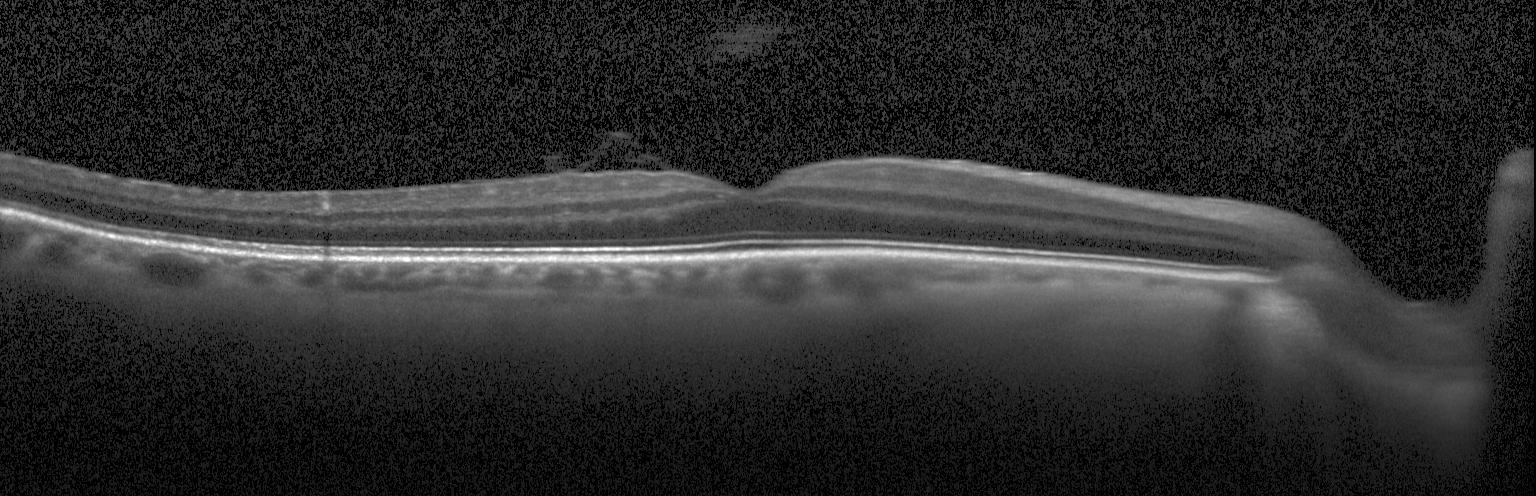

Spectral-domain optical coherence tomography; centered on the fovea; instrument: Heidelberg Spectralis; OCT B-scan. This B-scan demonstrates no CNV, no DME, and no drusen.